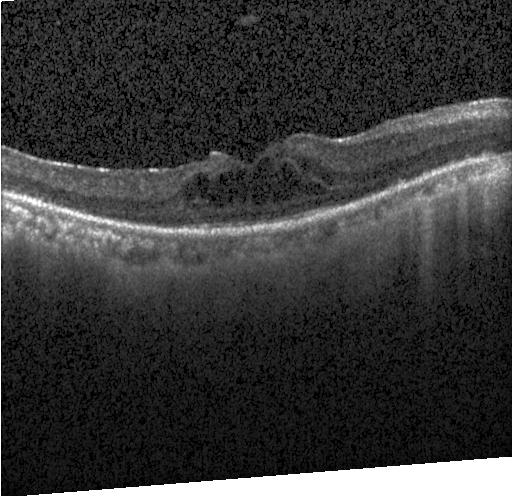

Retinal OCT B-scan.
DME.